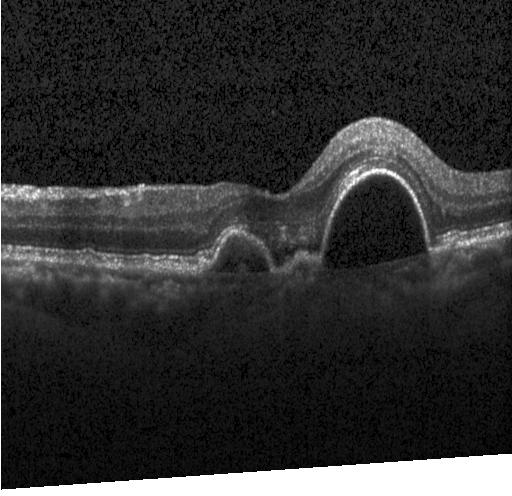 The scan shows a choroidal neovascular membrane.